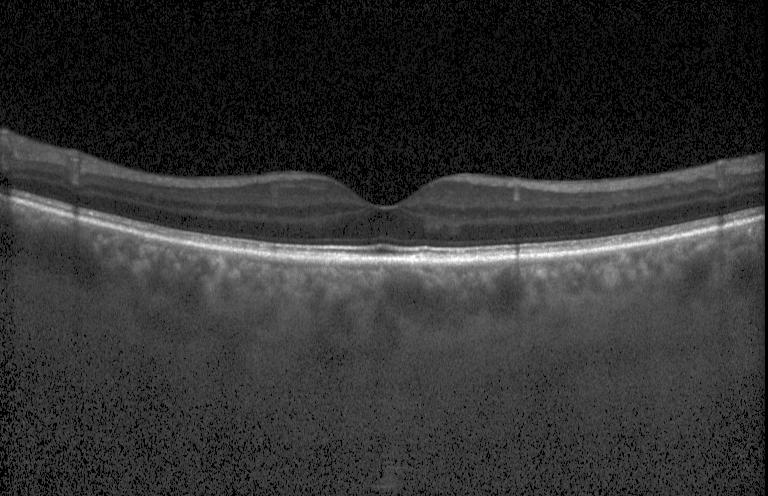
This B-scan demonstrates neither choroidal neovascularization, diabetic macular edema, nor drusen.